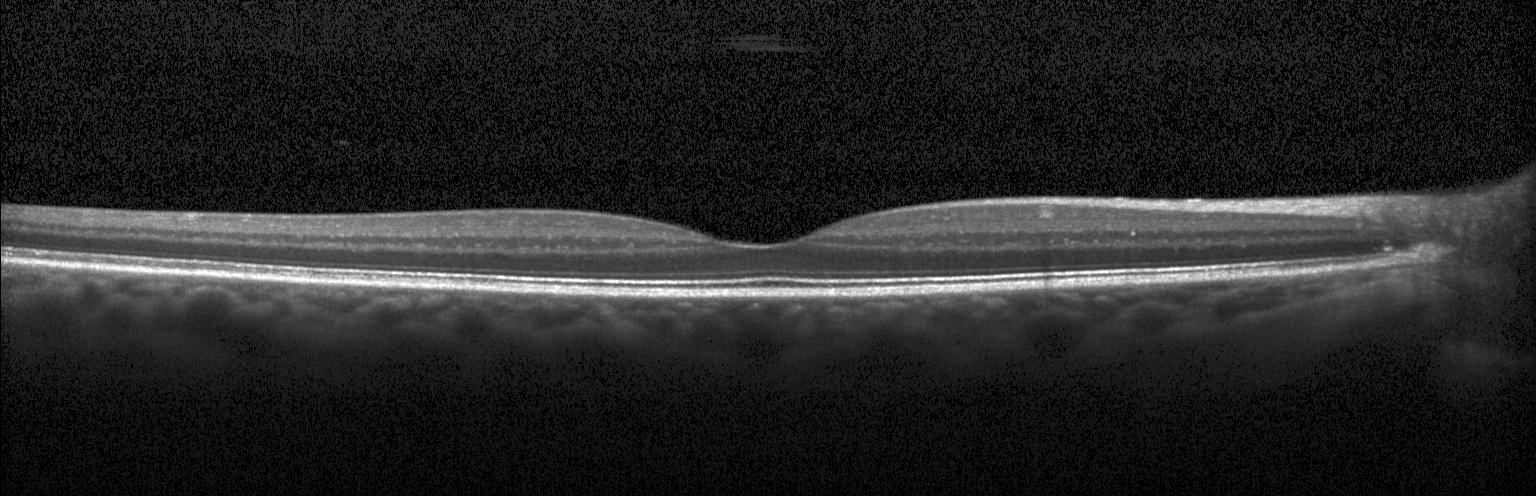 Retinal OCT B-scan, spectral-domain optical coherence tomography — Finding: no evidence of CNV, DME, or drusen.